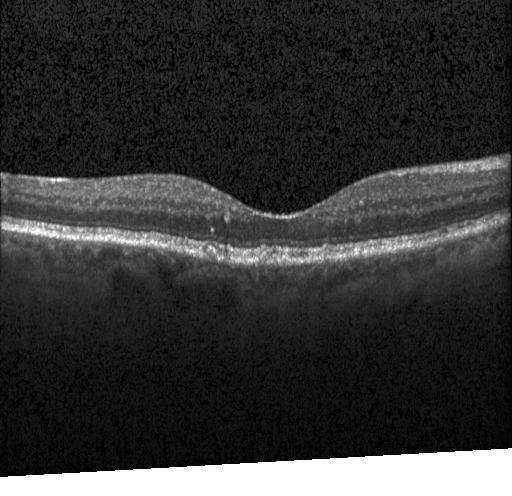 OCT line scan. Heidelberg Spectralis
Multiple drusen.